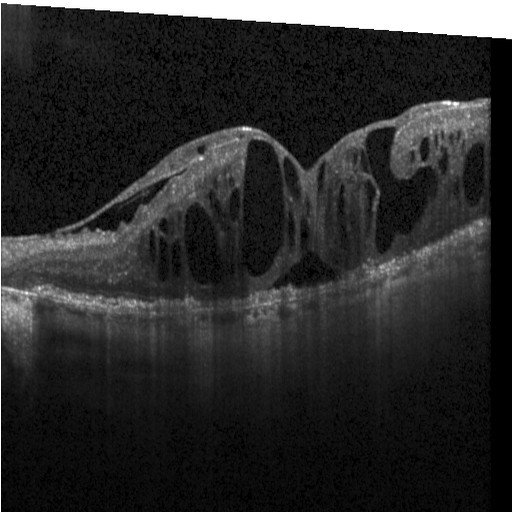
Optical coherence tomography scan.
Assessment: DME.